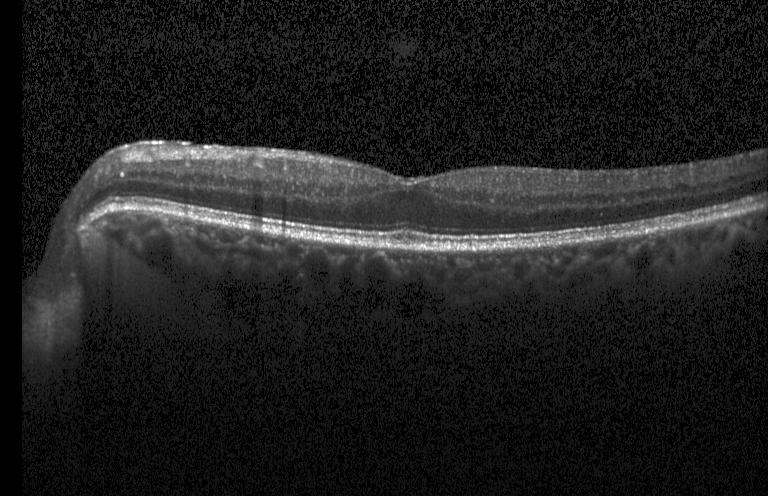 Heidelberg Spectralis OCT system · optical coherence tomography B-scan · SD-OCT
Diagnosis: no CNV, no DME, and no drusen.